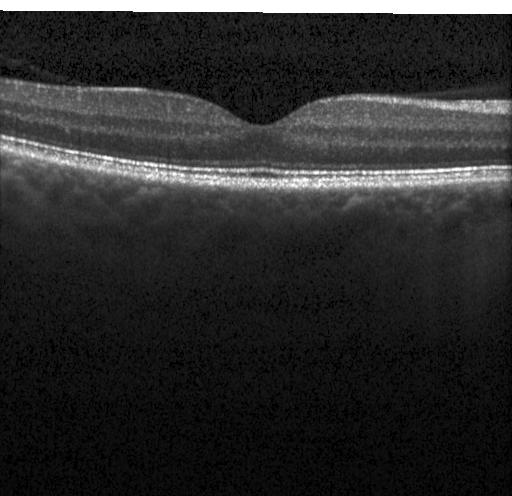

OCT B-scan showing no choroidal neovascularization, no diabetic macular edema, and no drusen.